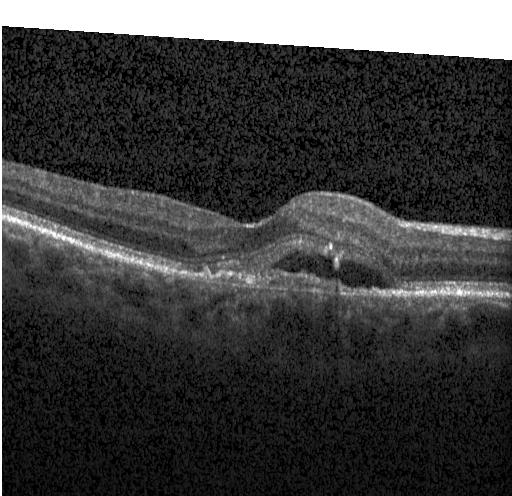

Impression: choroidal neovascularization.